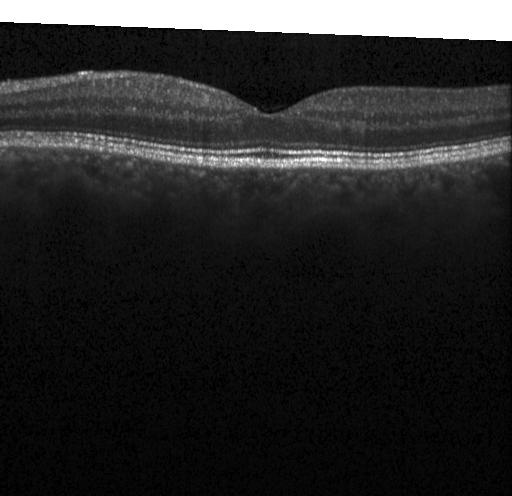 Macular OCT: no evidence of choroidal neovascularization, diabetic macular edema, or drusen.